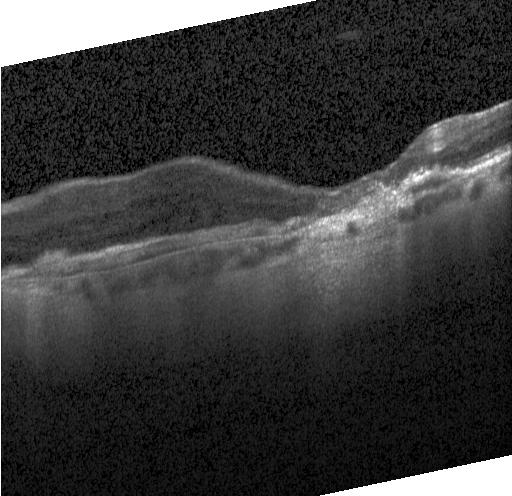
Finding: choroidal neovascularization (CNV).